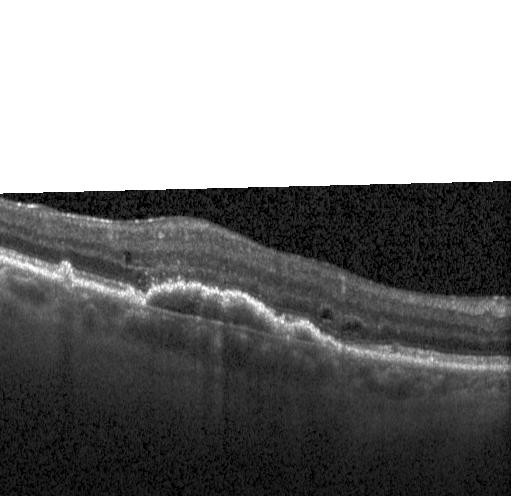
Finding: choroidal neovascularization (CNV).